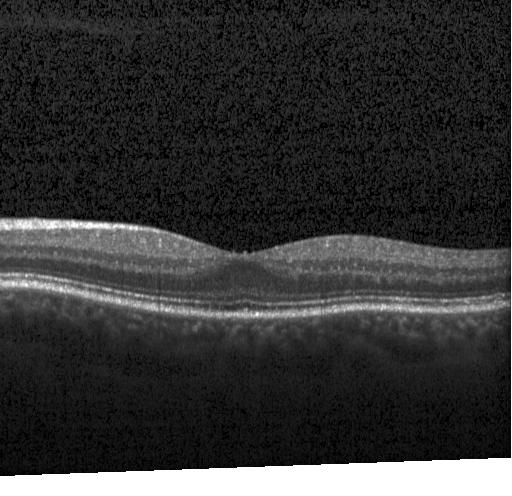

Spectral-domain optical coherence tomography, retinal OCT cross-section, centered on the fovea. Diagnosis: no CNV, no DME, and no drusen.